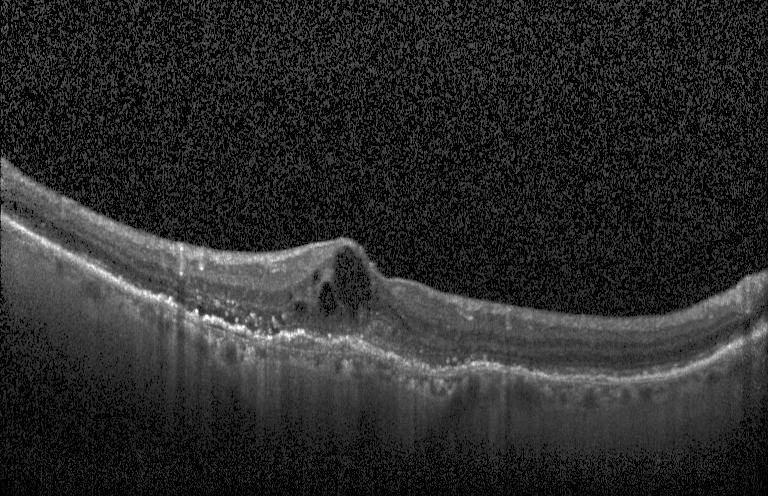

Retinal OCT cross-section. Centered on the fovea. Instrument: Heidelberg Spectralis. Spectral-domain OCT
Diagnosis: choroidal neovascularization (CNV).